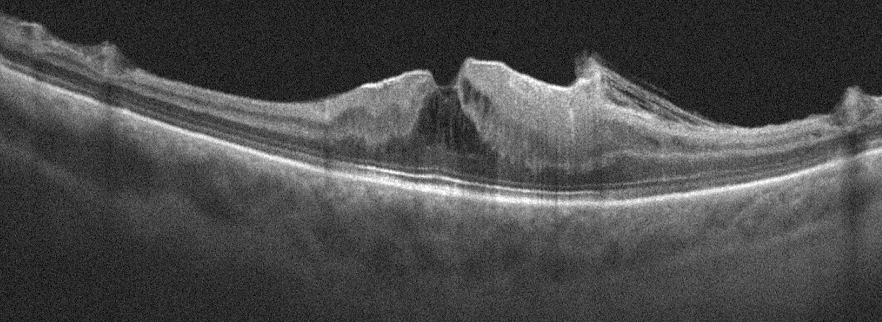

Macular scan; oculus dexter; retinal OCT B-scan; Optovue Avanti RTVue XR
Epiretinal membrane (ERM).